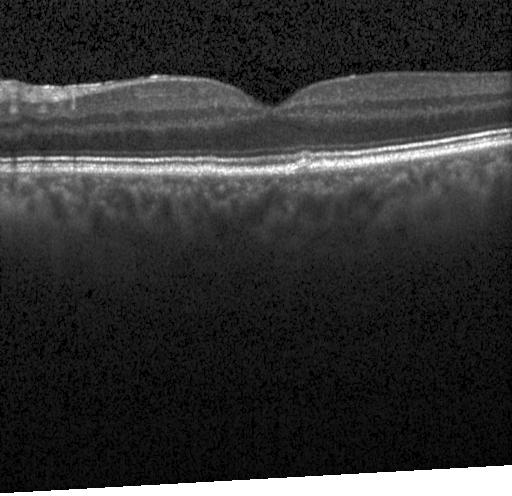
OCT line scan · spectral-domain OCT
Impression: drusen.